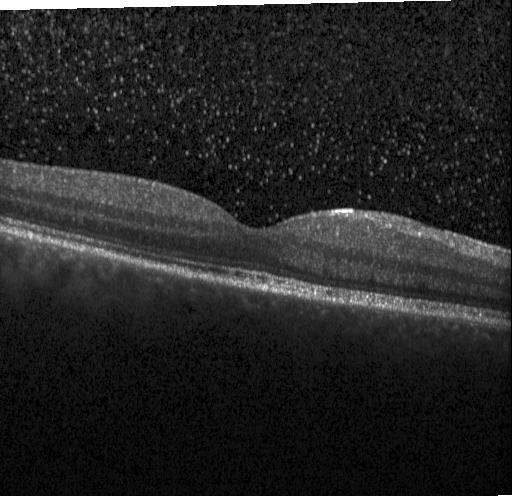 Retinal OCT cross-section, instrument: Heidelberg Spectralis — Diagnosis: no choroidal neovascularization, no diabetic macular edema, and no drusen.